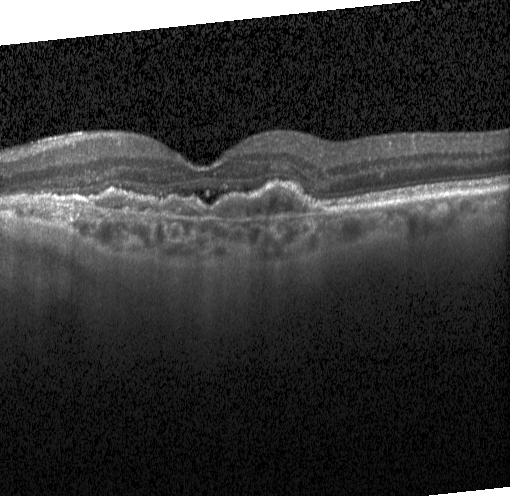
OCT finding: choroidal neovascularization.